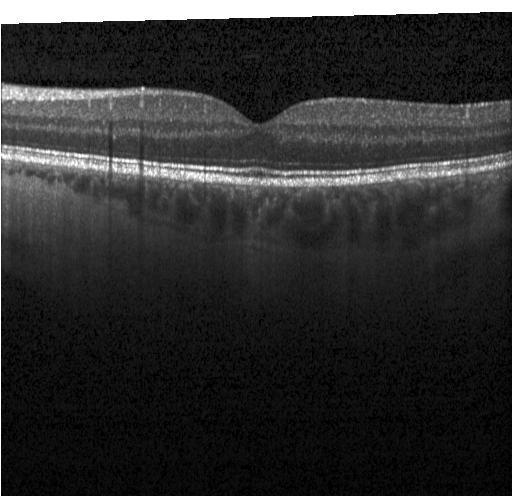

Centered on the fovea · Heidelberg Spectralis · optical coherence tomography scan. Macular OCT: no choroidal neovascularization, no diabetic macular edema, and no drusen.